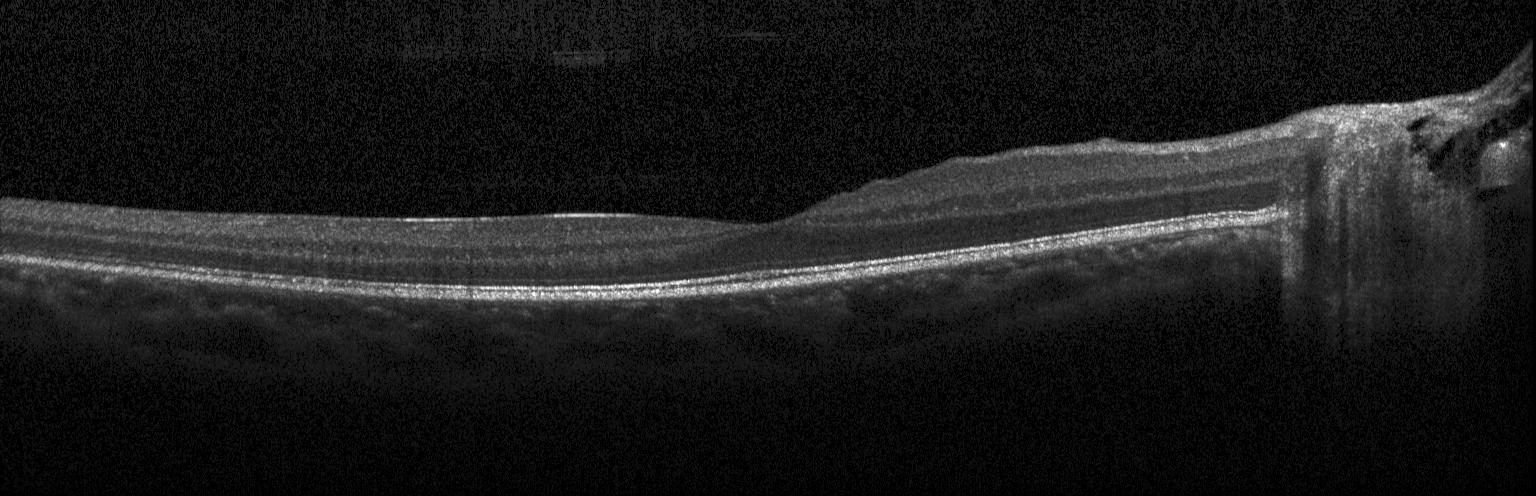

Optical coherence tomography scan. Instrument: Heidelberg Spectralis. Centered on the fovea.
Macular OCT: no evidence of choroidal neovascularization, diabetic macular edema, or drusen.